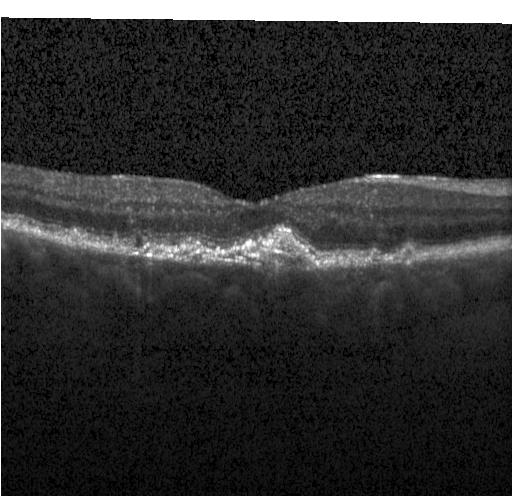
OCT line scan
Assessment: a choroidal neovascular membrane.